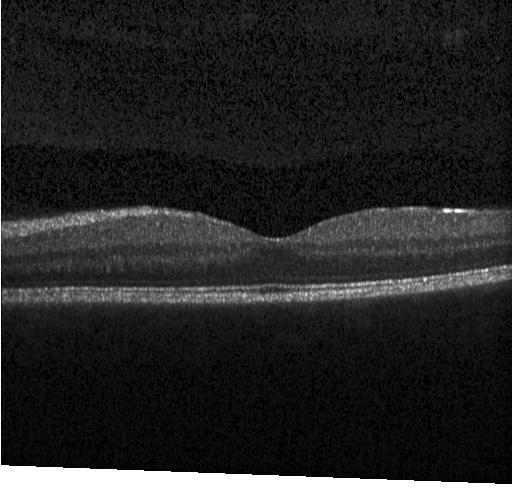 Macular scan. Heidelberg Spectralis OCT system. OCT line scan
This B-scan demonstrates no choroidal neovascularization, diabetic macular edema, or drusen.